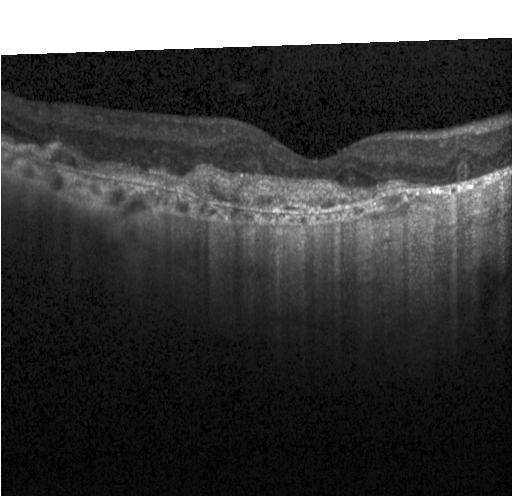

OCT finding: a choroidal neovascular membrane.